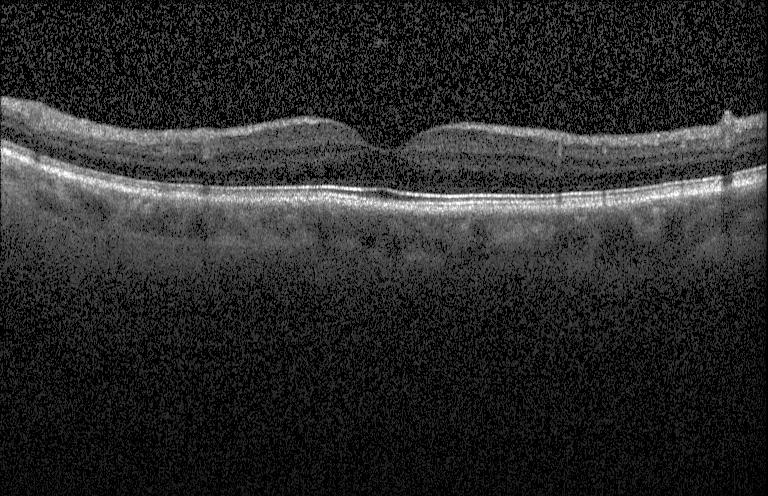 OCT line scan. Acquired on a Heidelberg Spectralis. Fovea-centered. Spectral-domain optical coherence tomography
Assessment: neither CNV, DME, nor drusen.